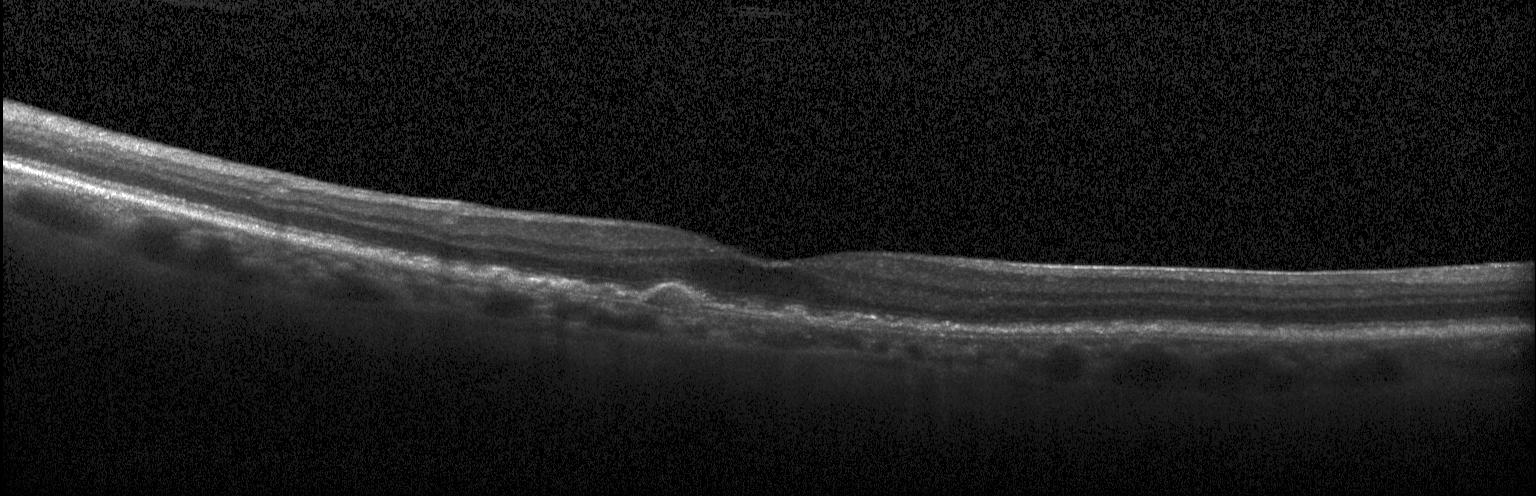

OCT line scan
Impression: drusen.